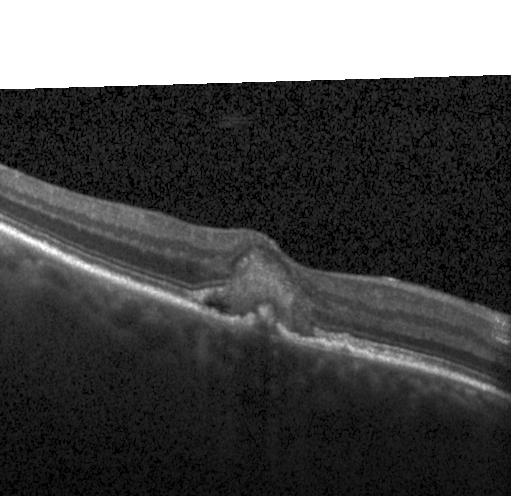 The scan shows a choroidal neovascular membrane.